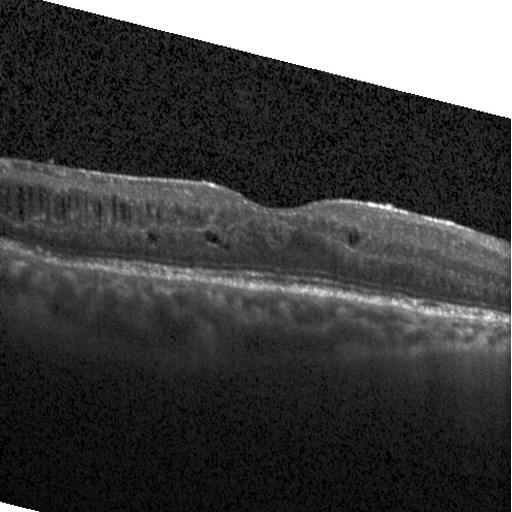
Spectral-domain OCT. Acquired on a Heidelberg Spectralis. OCT line scan. Macular scan — Diagnosis: diabetic macular edema.